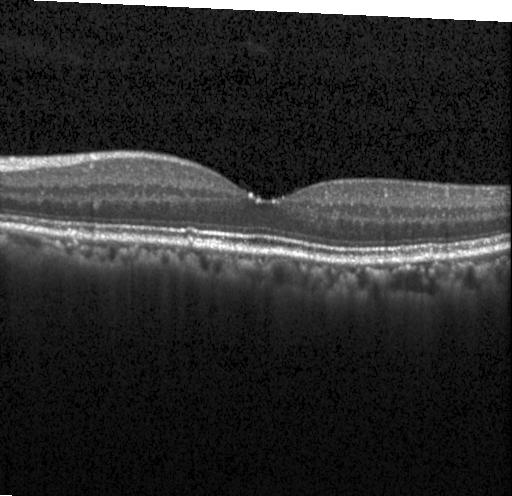
Acquired on a Heidelberg Spectralis. Macular scan. OCT line scan. Spectral-domain OCT. Diagnosis: neither choroidal neovascularization, diabetic macular edema, nor drusen.